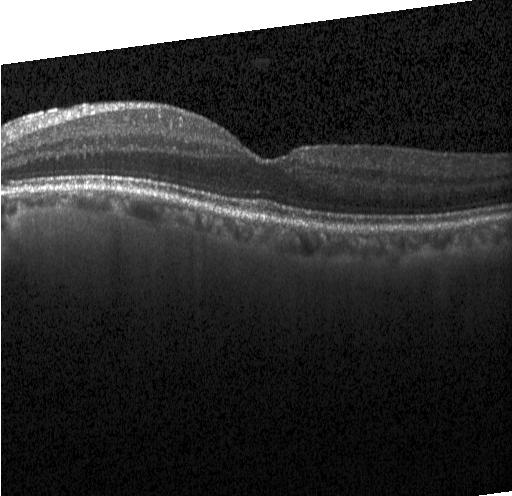 OCT B-scan. Spectral-domain OCT. Horizontal scan through the fovea. Heidelberg Spectralis OCT system — Diagnosis: no choroidal neovascularization, no diabetic macular edema, and no drusen.